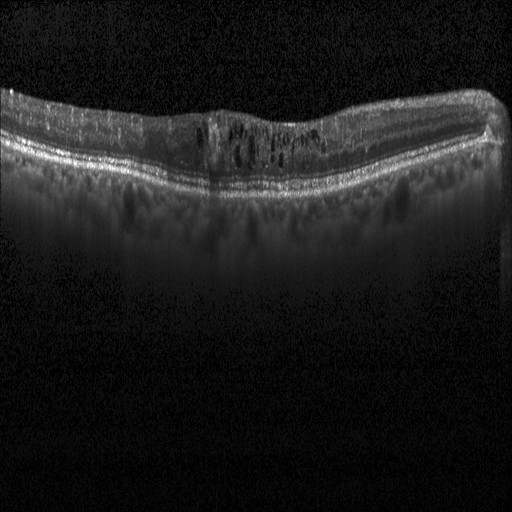
Macular OCT: diabetic macular edema (DME).